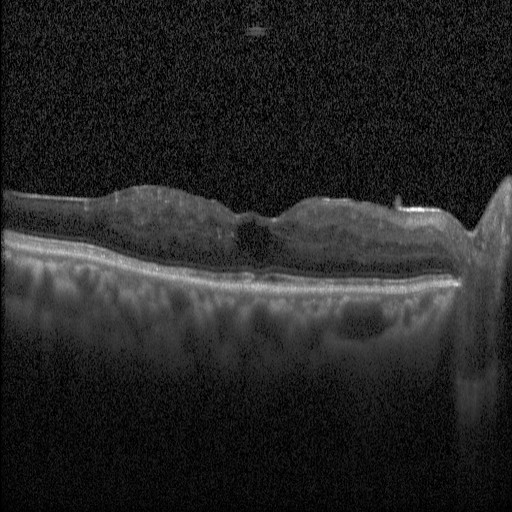

Fovea-centered; instrument: Heidelberg Spectralis; OCT B-scan; spectral-domain optical coherence tomography.
Impression: diabetic macular edema.